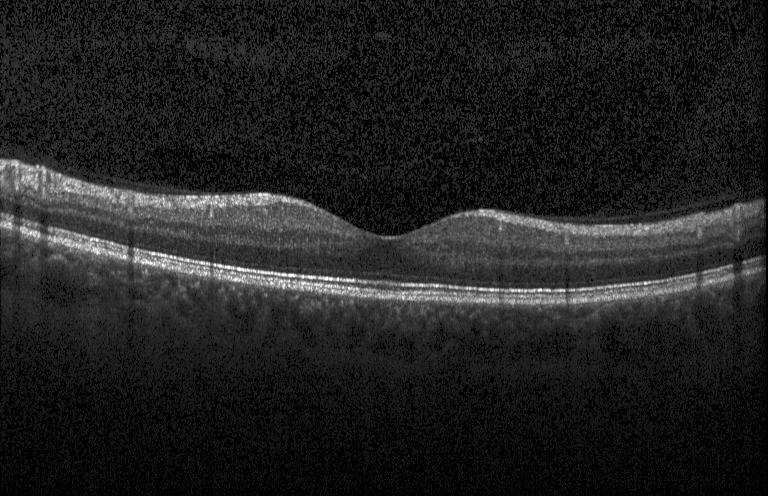 Optical coherence tomography B-scan · spectral-domain optical coherence tomography · fovea-centered · Heidelberg Spectralis OCT system
Dx: neither choroidal neovascularization, diabetic macular edema, nor drusen.